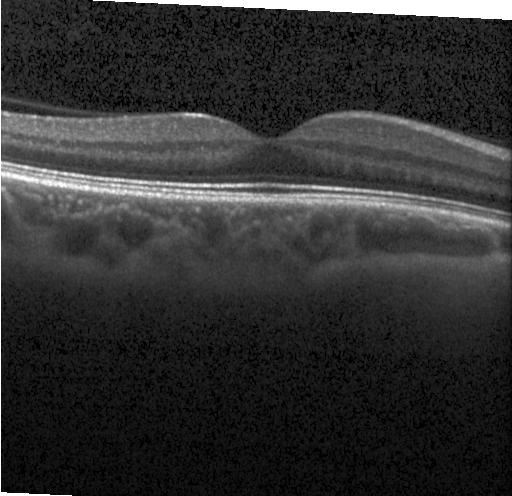 Horizontal scan through the fovea, SD-OCT, OCT B-scan, Heidelberg Spectralis.
Dx: neither CNV, DME, nor drusen.